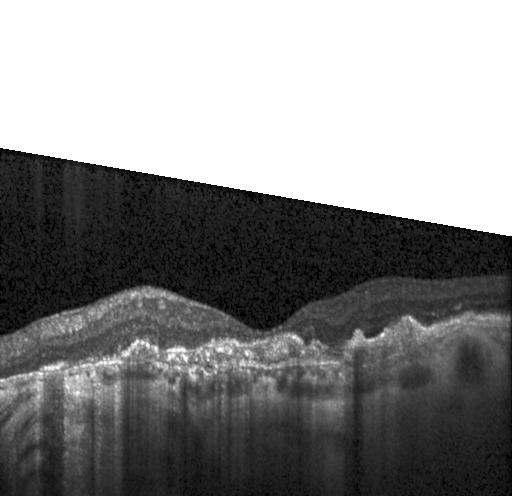

Finding: a choroidal neovascular membrane.